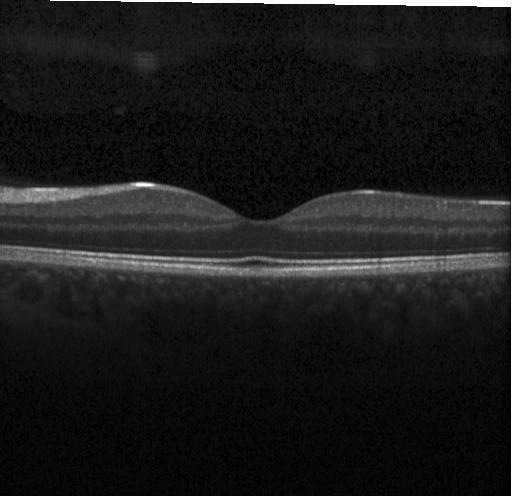
Optical coherence tomography B-scan. Spectral-domain OCT. Fovea-centered
Assessment: neither choroidal neovascularization, diabetic macular edema, nor drusen.